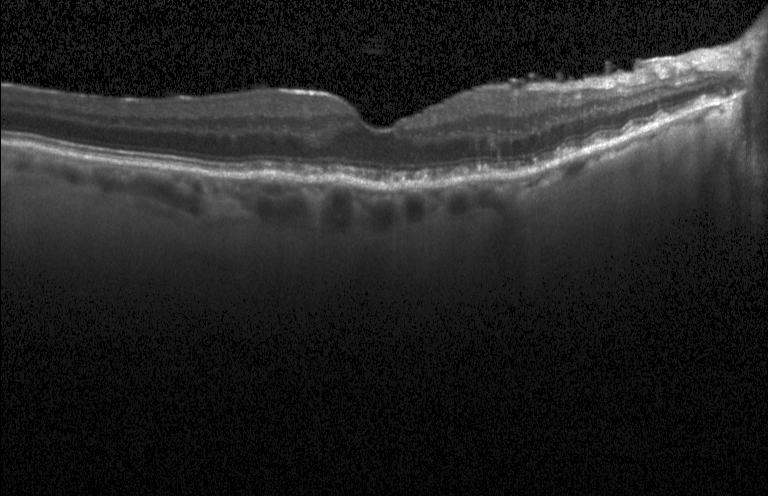

Diagnosis: multiple drusen.